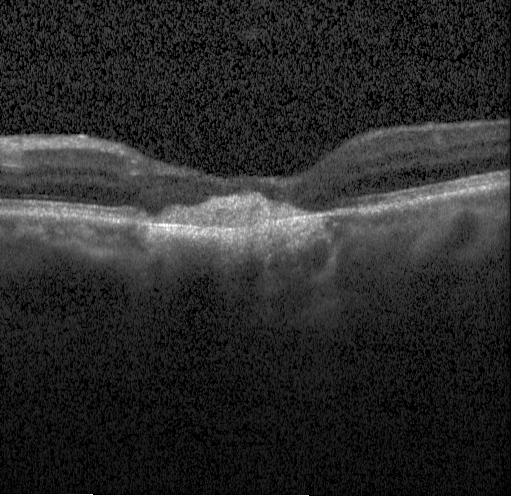 Through the macula. Optical coherence tomography scan. Heidelberg Spectralis OCT system
Dx: a choroidal neovascular membrane.